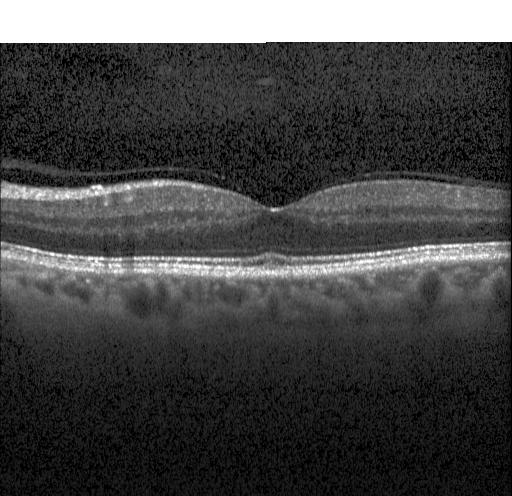
Dx: neither choroidal neovascularization, diabetic macular edema, nor drusen.